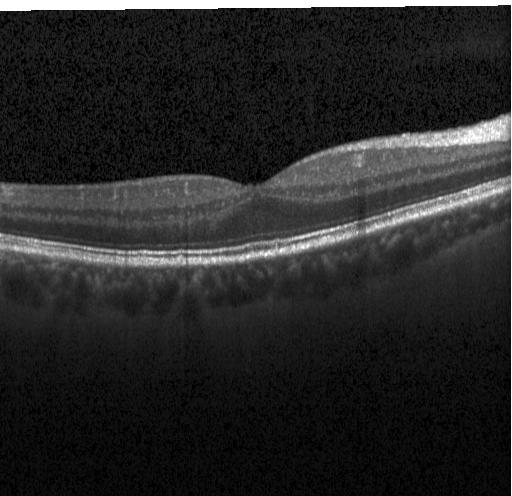
Retinal OCT cross-section showing no CNV, no DME, and no drusen.